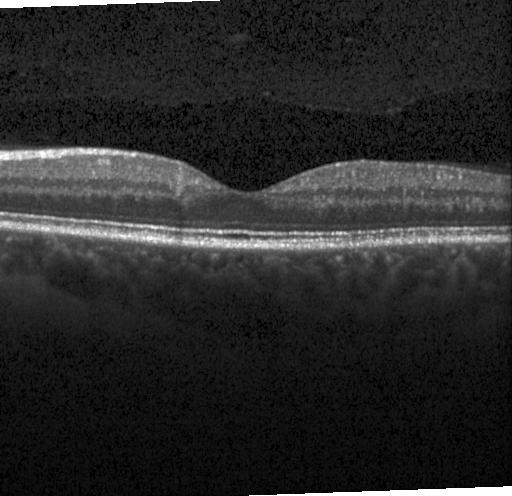 Optical coherence tomography scan · fovea-centered. Impression: no evidence of choroidal neovascularization, diabetic macular edema, or drusen.